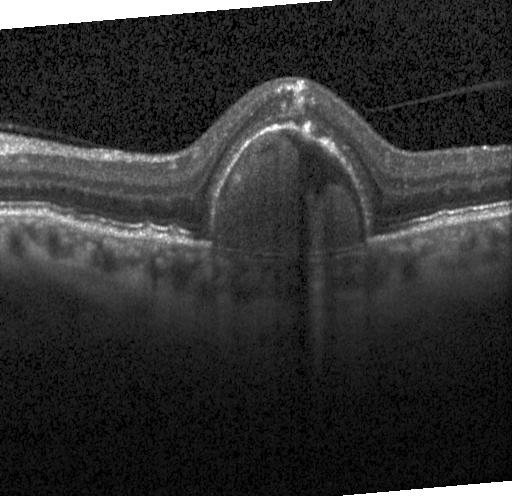
Optical coherence tomography scan, SD-OCT, Heidelberg Spectralis OCT system, through the macula — Macular OCT: a choroidal neovascular membrane.